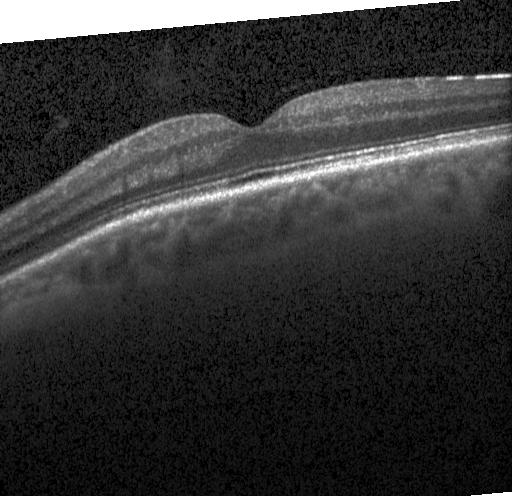 Diagnosis: neither choroidal neovascularization, diabetic macular edema, nor drusen.